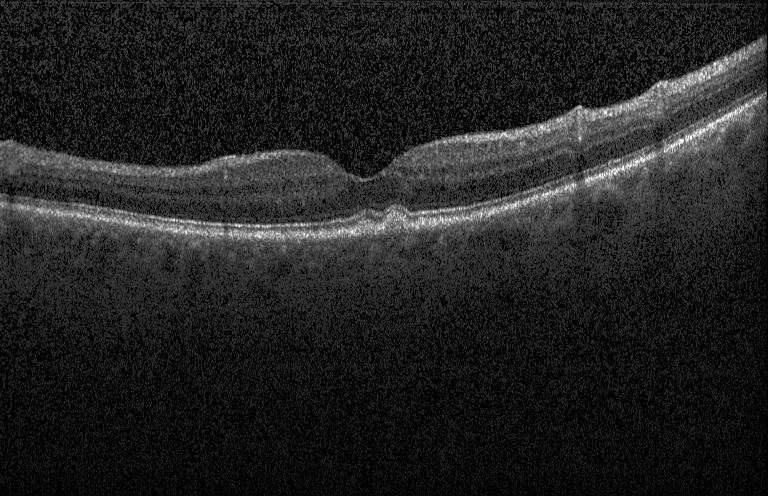

Optical coherence tomography scan.
Drusen.